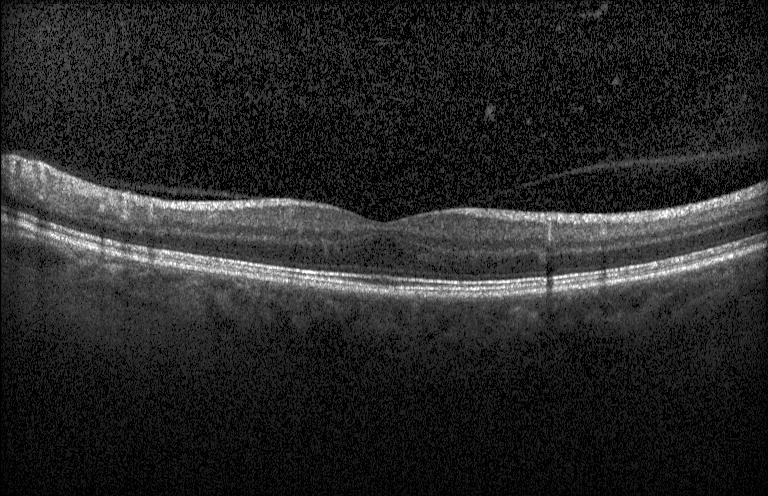 Spectral-domain optical coherence tomography, OCT line scan — Finding: no evidence of choroidal neovascularization, diabetic macular edema, or drusen.